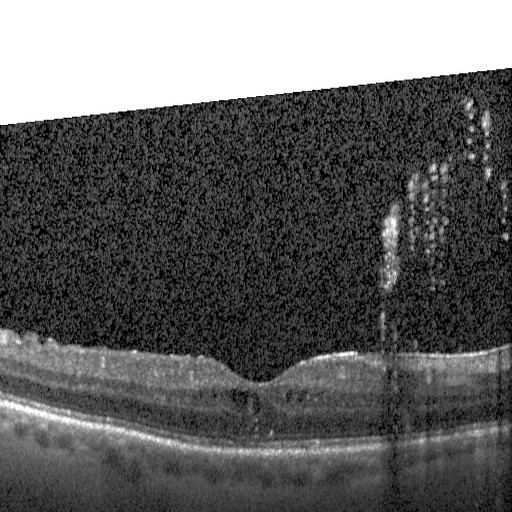

Optical coherence tomography B-scan. Finding: DME.